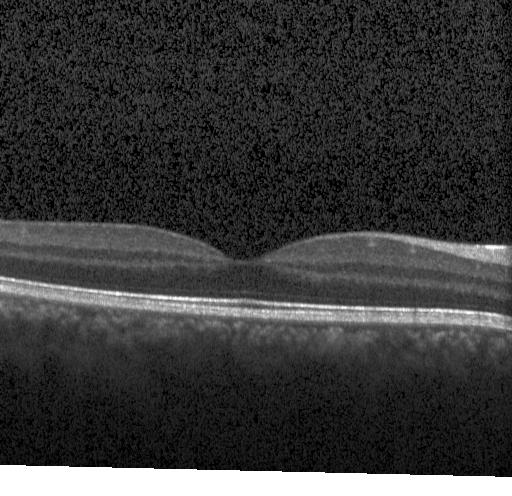 Retinal OCT B-scan · spectral-domain optical coherence tomography · instrument: Heidelberg Spectralis · macular scan
Impression: no choroidal neovascularization, no diabetic macular edema, and no drusen.